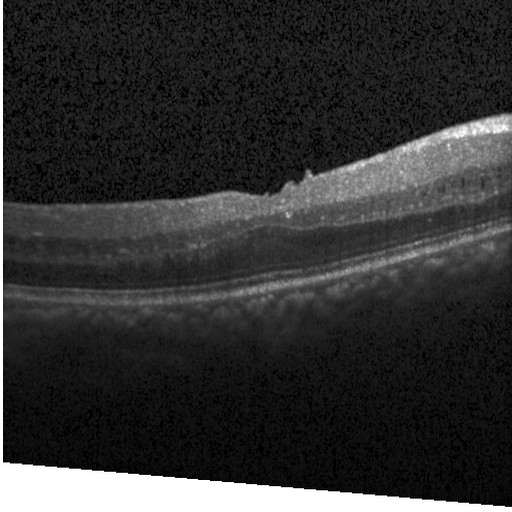
Impression: diabetic macular edema.